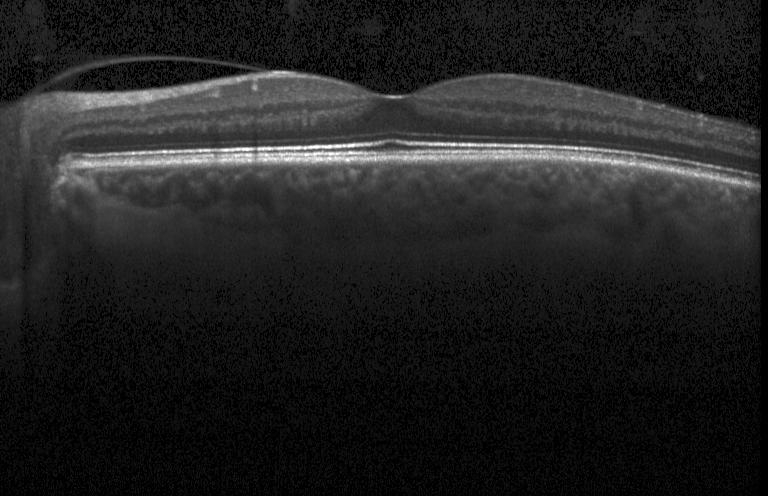 Assessment: neither CNV, DME, nor drusen.